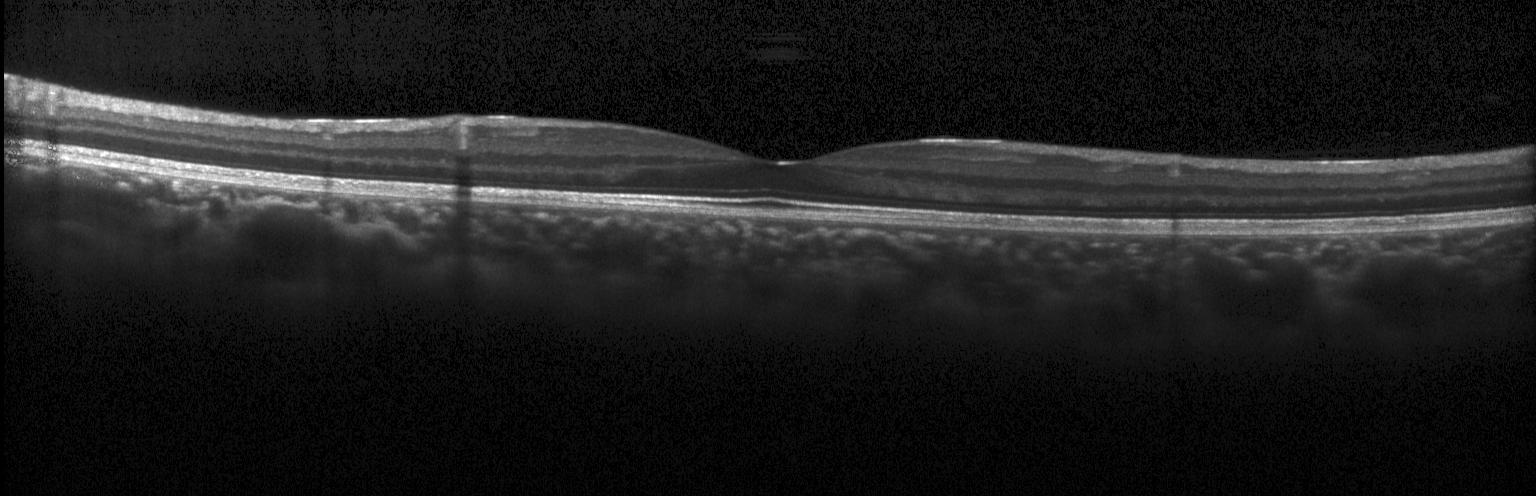 Centered on the fovea · Heidelberg Spectralis · retinal OCT B-scan
OCT finding: no choroidal neovascularization, no diabetic macular edema, and no drusen.